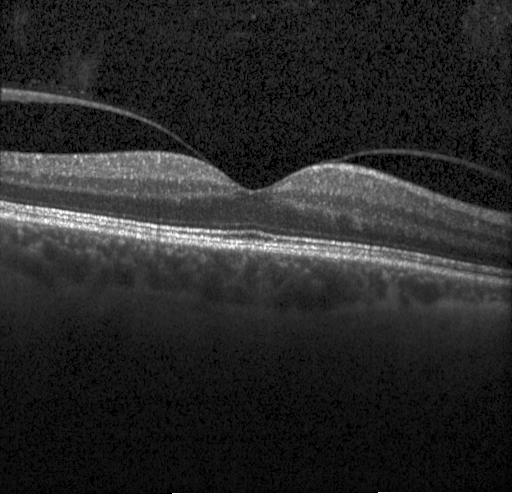 Macular OCT: neither choroidal neovascularization, diabetic macular edema, nor drusen.